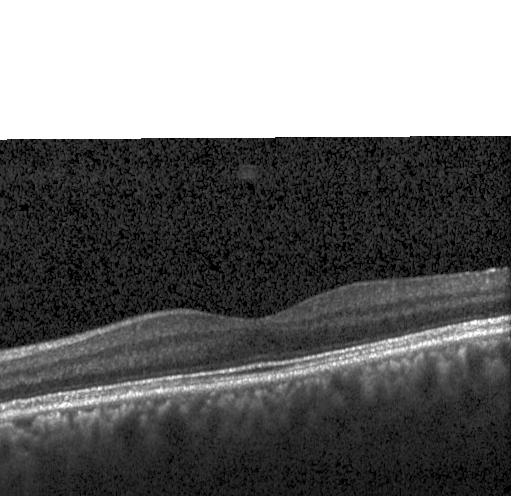 Diagnosis: no choroidal neovascularization, diabetic macular edema, or drusen.